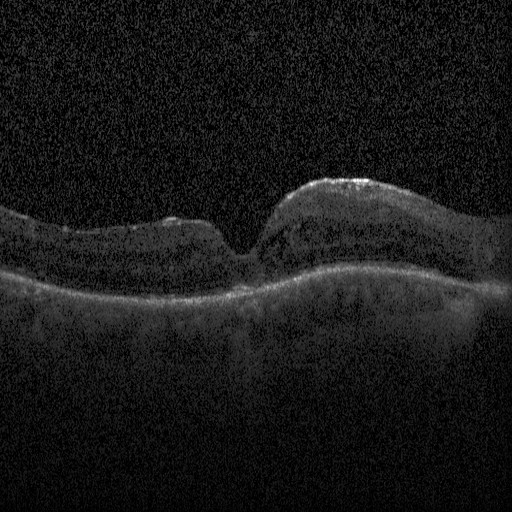

OCT finding: diabetic macular edema (DME).